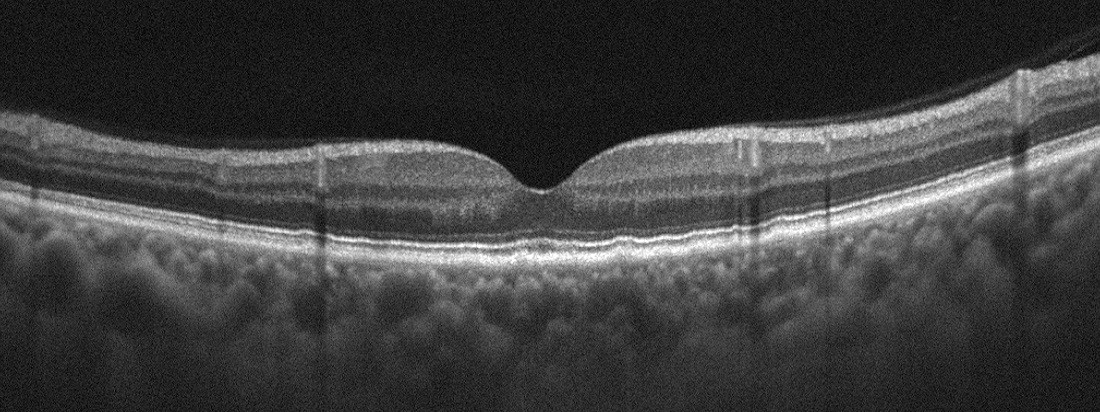
Instrument: Optovue Avanti RTVue XR · OCT B-scan · fovea-centered. Finding: age-related macular degeneration (AMD).